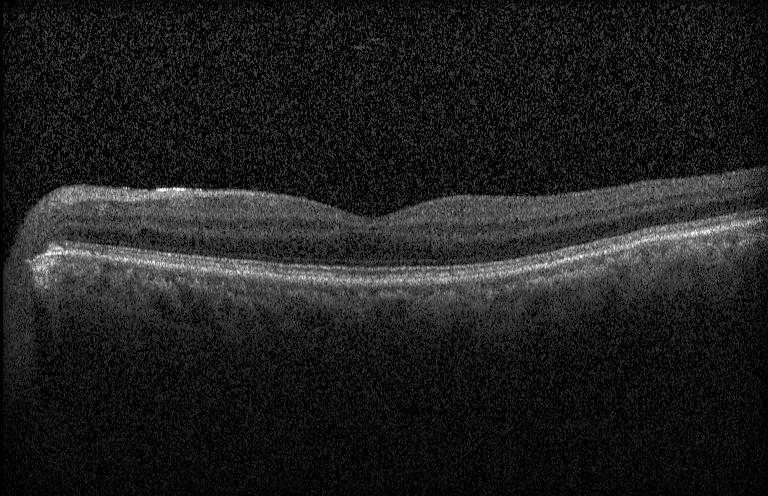
This B-scan demonstrates neither choroidal neovascularization, diabetic macular edema, nor drusen.